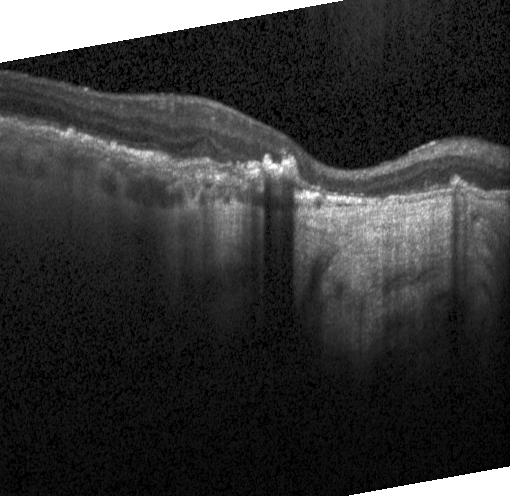 Optical coherence tomography scan, fovea-centered.
Impression: a choroidal neovascular membrane.